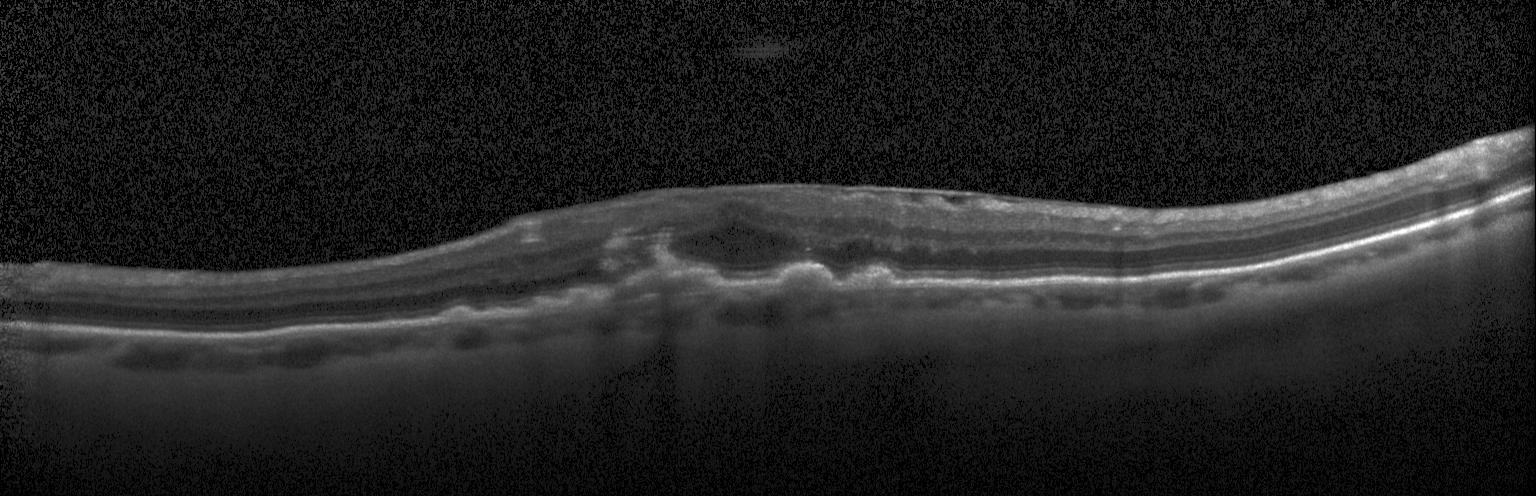
Spectral-domain OCT; optical coherence tomography scan. Impression: multiple drusen.